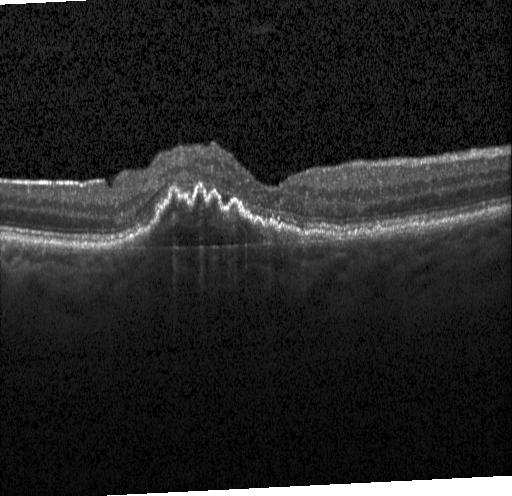
Retinal OCT cross-section — Impression: a choroidal neovascular membrane.